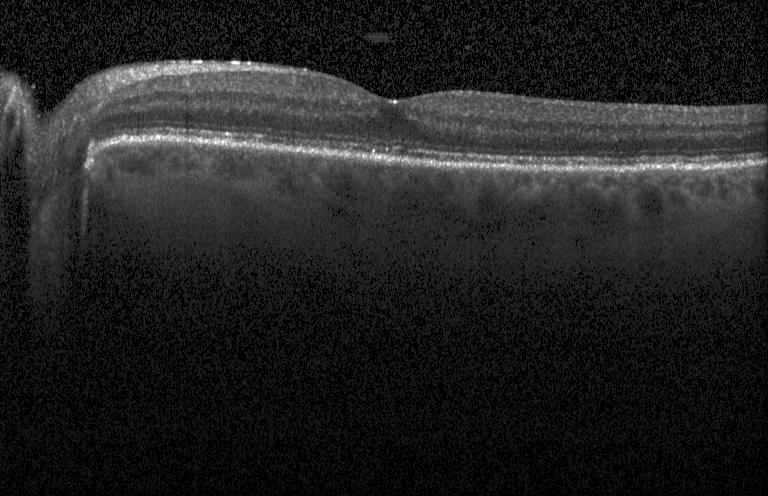

No evidence of choroidal neovascularization, diabetic macular edema, or drusen.